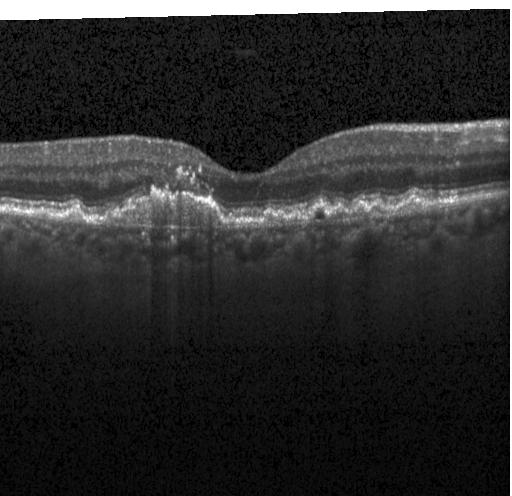
OCT scan showing choroidal neovascularization (CNV).